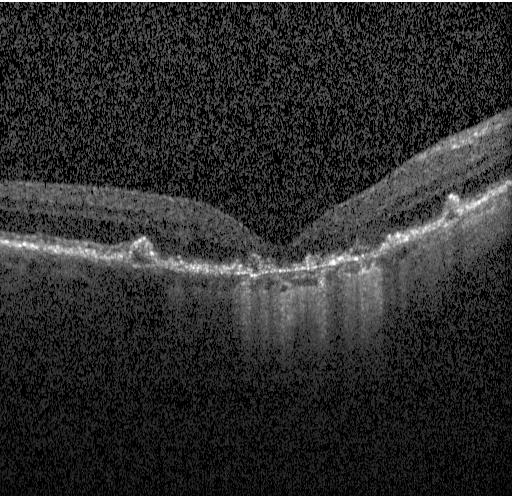 Dx: CNV.